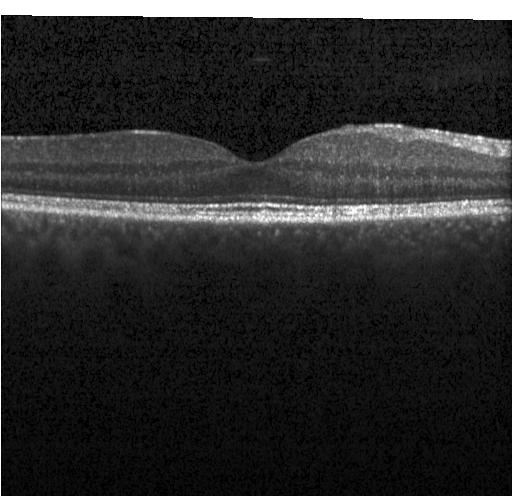

Retinal OCT B-scan.
Finding: no evidence of CNV, DME, or drusen.